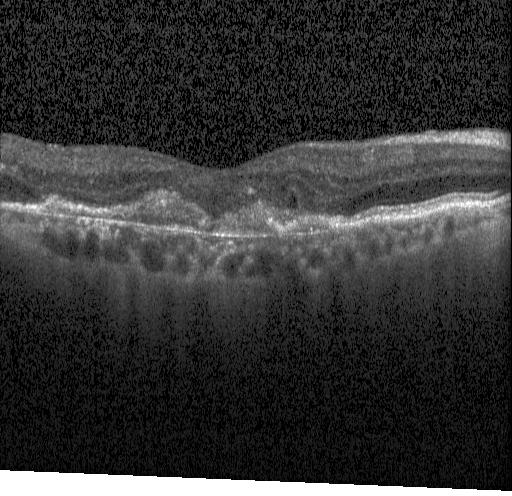 Acquired on a Heidelberg Spectralis · retinal OCT B-scan.
Finding: CNV.